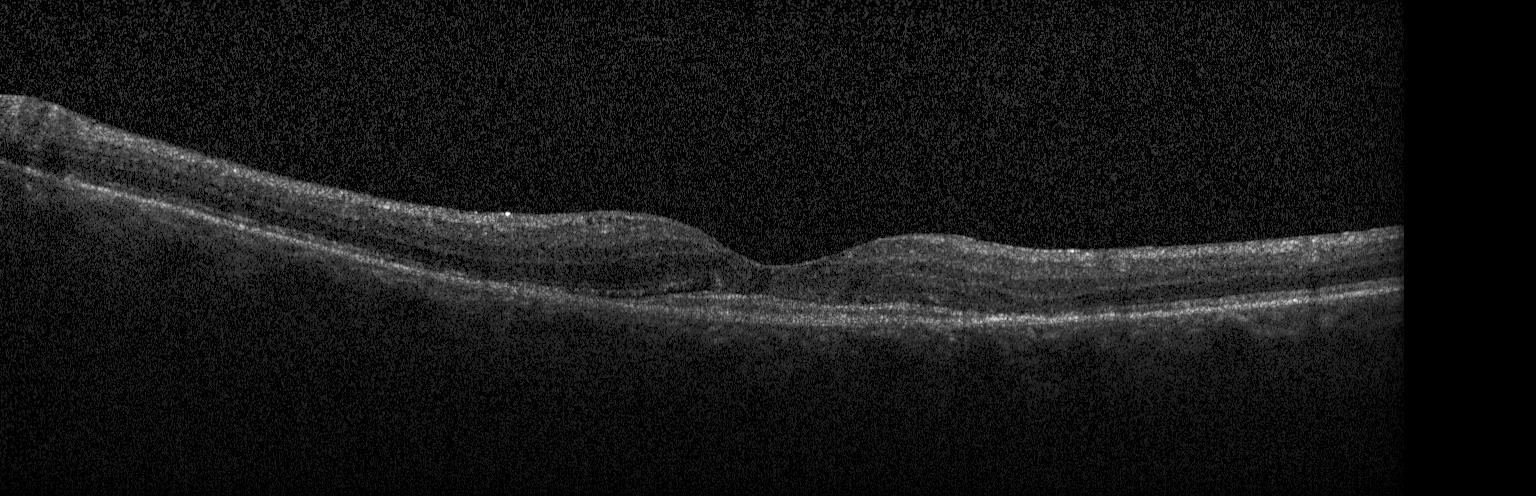 Spectral-domain OCT, optical coherence tomography B-scan
Impression: choroidal neovascularization (CNV).